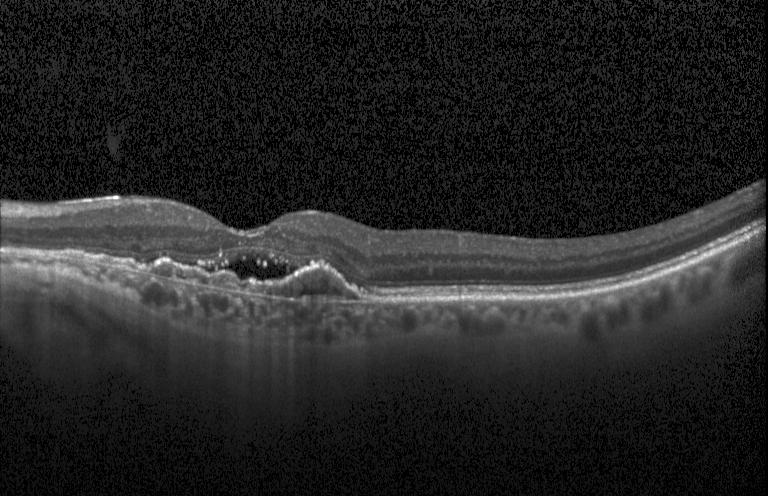

OCT finding: choroidal neovascularization.